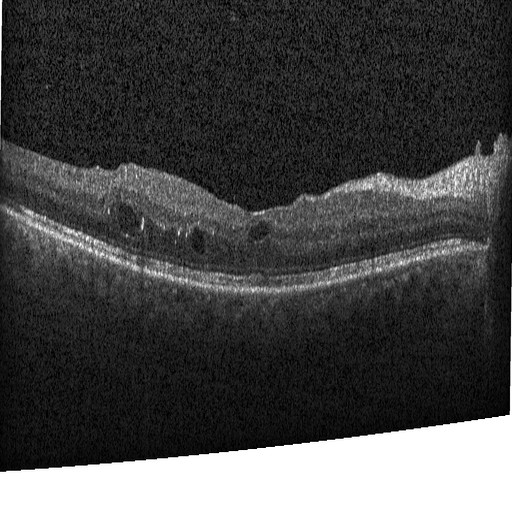
Optical coherence tomography B-scan. Assessment: diabetic macular edema.